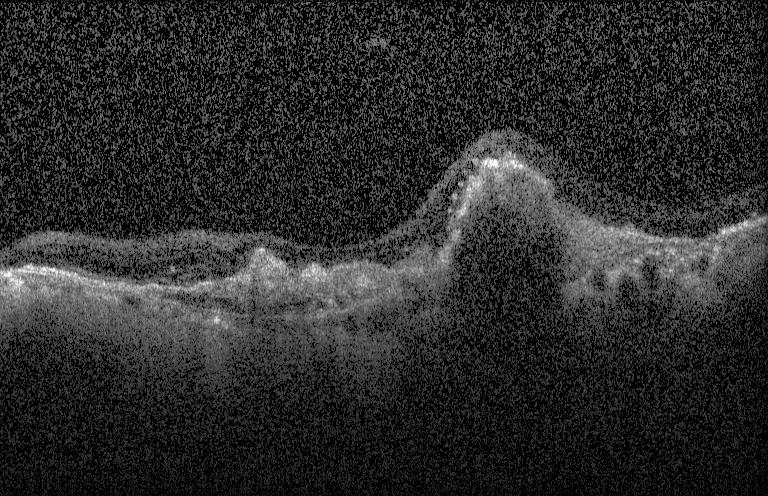 Optical coherence tomography B-scan. Macular scan. Assessment: a choroidal neovascular membrane.